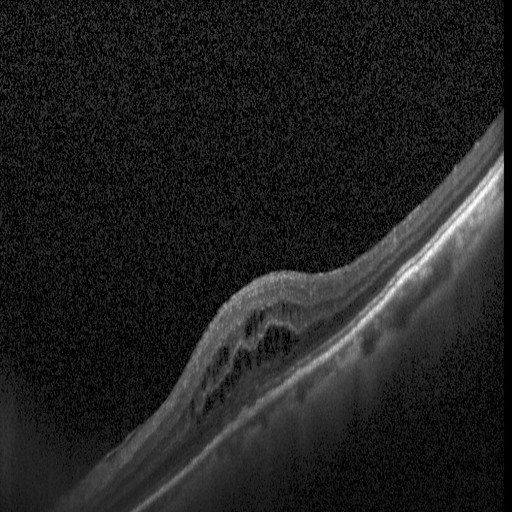
Spectral-domain OCT; instrument: Heidelberg Spectralis; OCT line scan — Impression: DME.